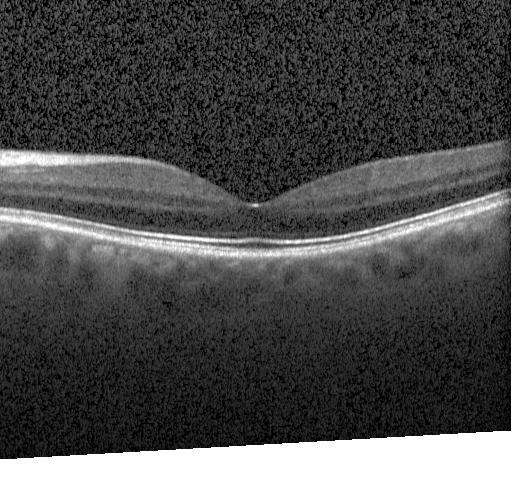 The scan shows no choroidal neovascularization, diabetic macular edema, or drusen.